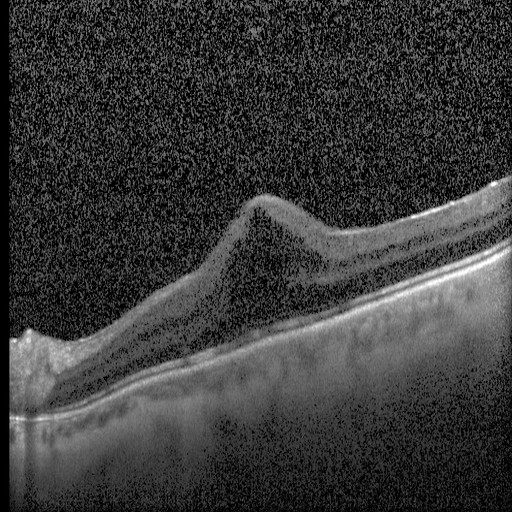
OCT finding: diabetic macular edema (DME).